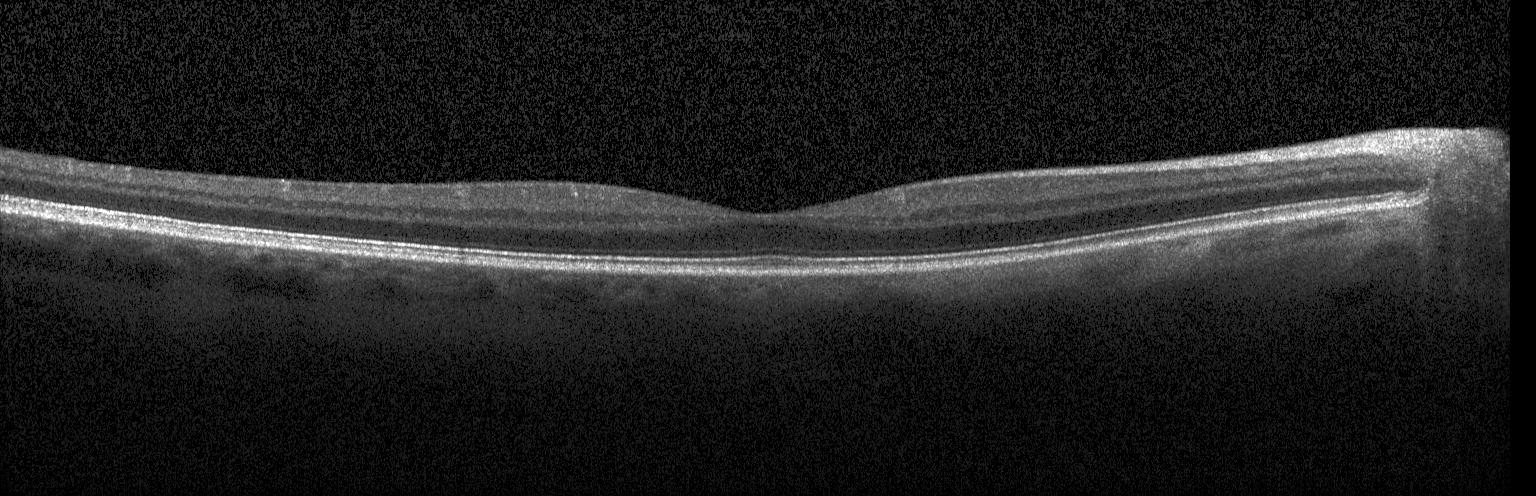
Optical coherence tomography scan
Dx: neither CNV, DME, nor drusen.